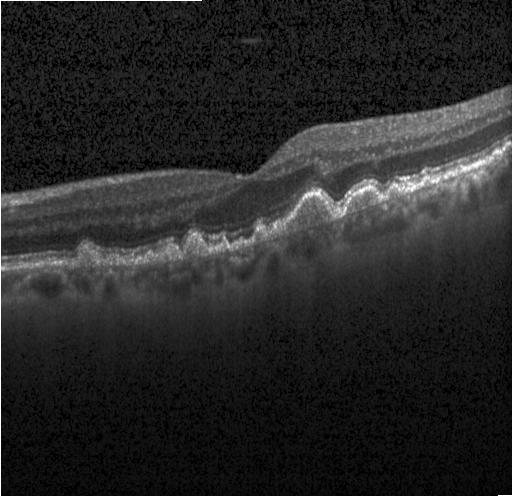
Retinal OCT cross-section showing sub-RPE drusenoid deposits.